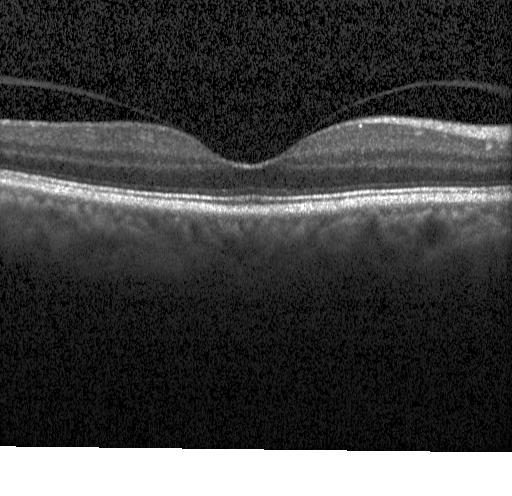
Centered on the fovea. Retinal OCT cross-section
Macular OCT: neither CNV, DME, nor drusen.